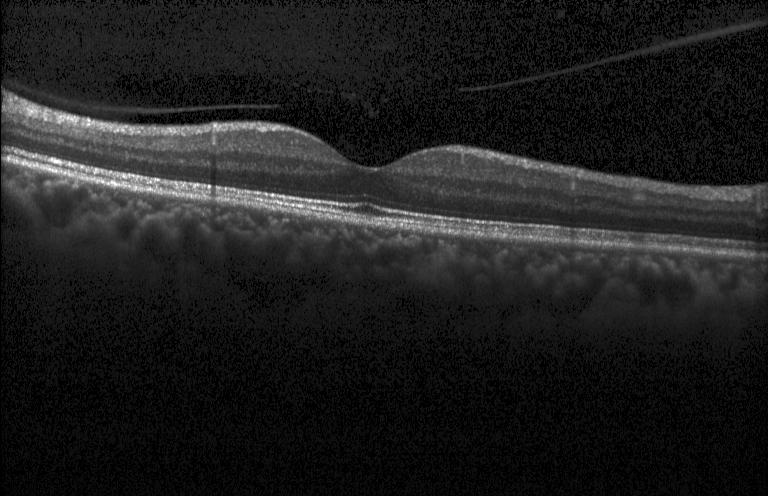
Horizontal scan through the fovea. Optical coherence tomography scan. Acquired on a Heidelberg Spectralis — Diagnosis: no choroidal neovascularization, no diabetic macular edema, and no drusen.